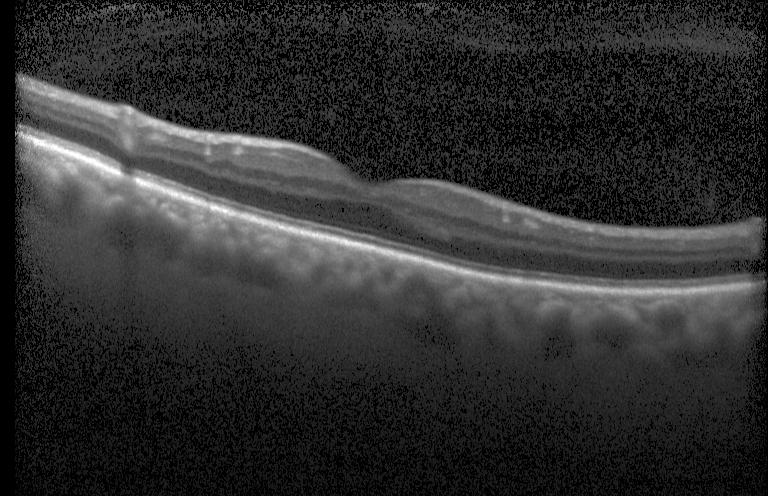 SD-OCT; retinal OCT cross-section.
Diagnosis: neither choroidal neovascularization, diabetic macular edema, nor drusen.